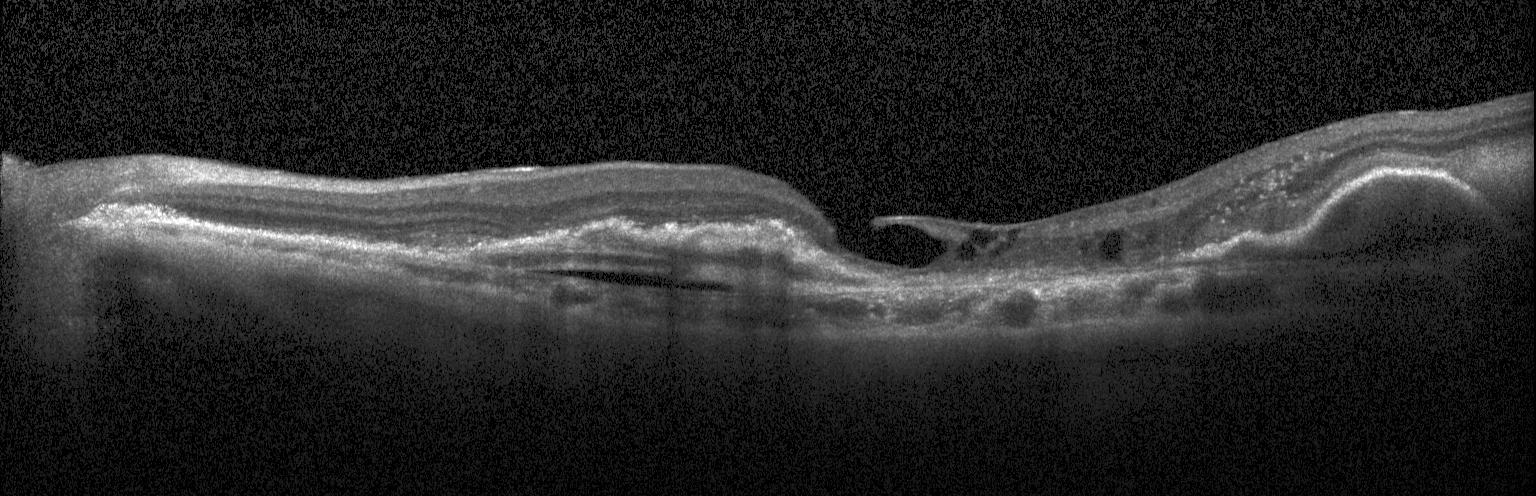

Horizontal scan through the fovea. Acquired on a Heidelberg Spectralis. Optical coherence tomography B-scan. Macular OCT: choroidal neovascularization.